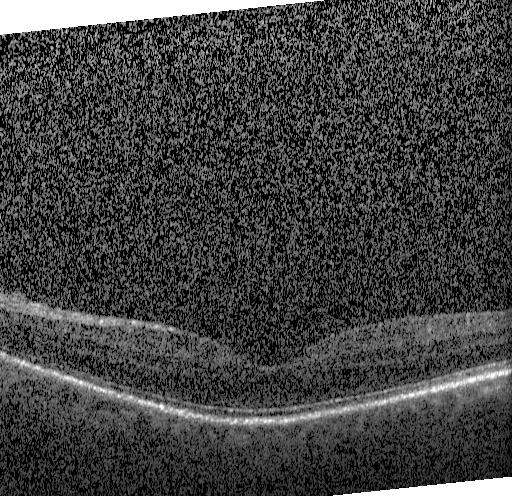

Acquired on a Heidelberg Spectralis · retinal OCT B-scan — OCT finding: no evidence of choroidal neovascularization, diabetic macular edema, or drusen.